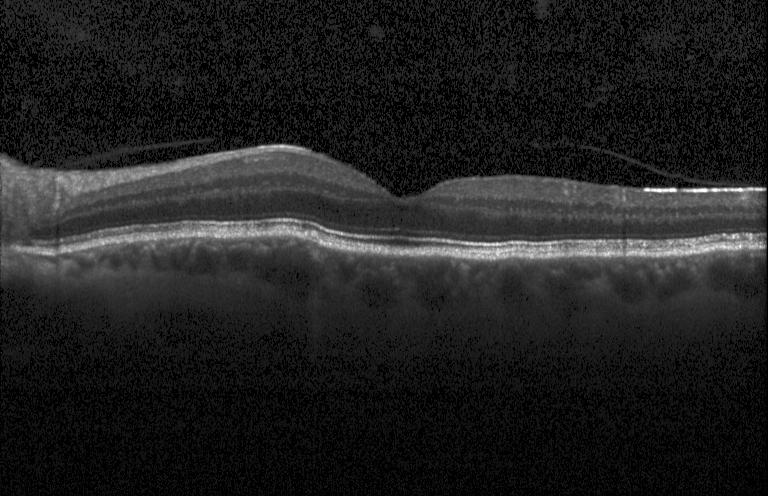
Through the macula · instrument: Heidelberg Spectralis · optical coherence tomography scan
Impression: neither choroidal neovascularization, diabetic macular edema, nor drusen.